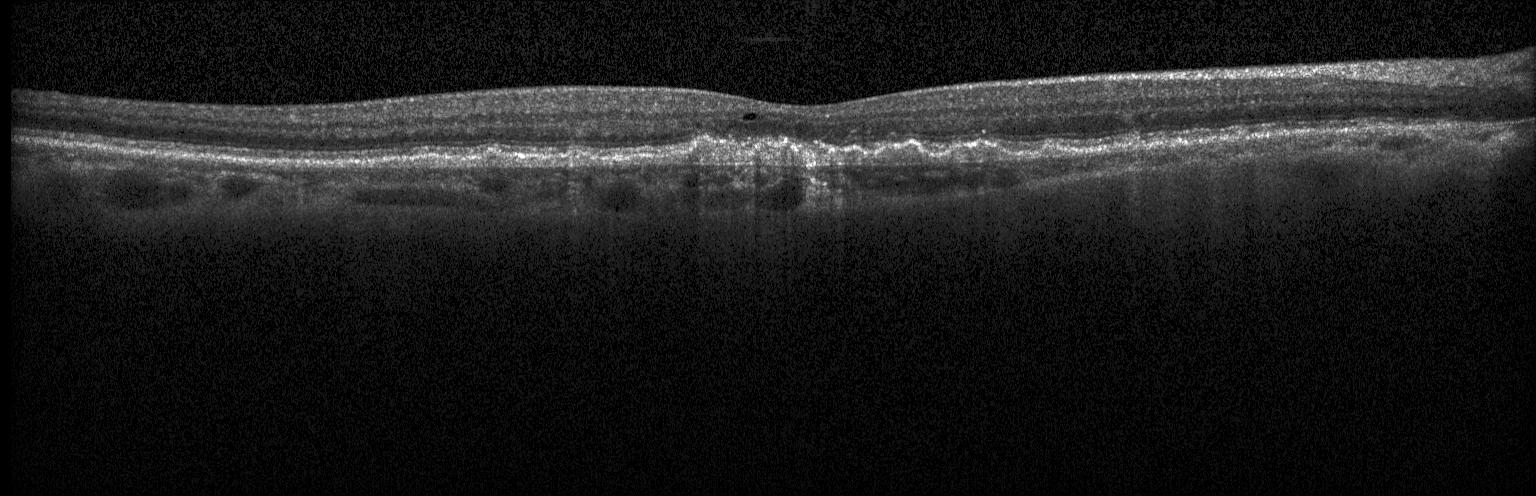 Diagnosis: a choroidal neovascular membrane.